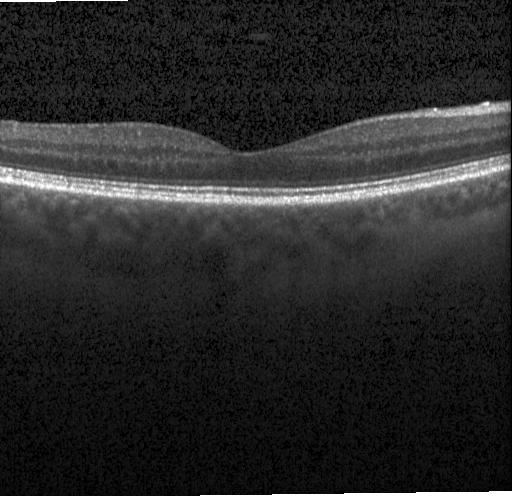 Retinal OCT cross-section.
Impression: no evidence of choroidal neovascularization, diabetic macular edema, or drusen.